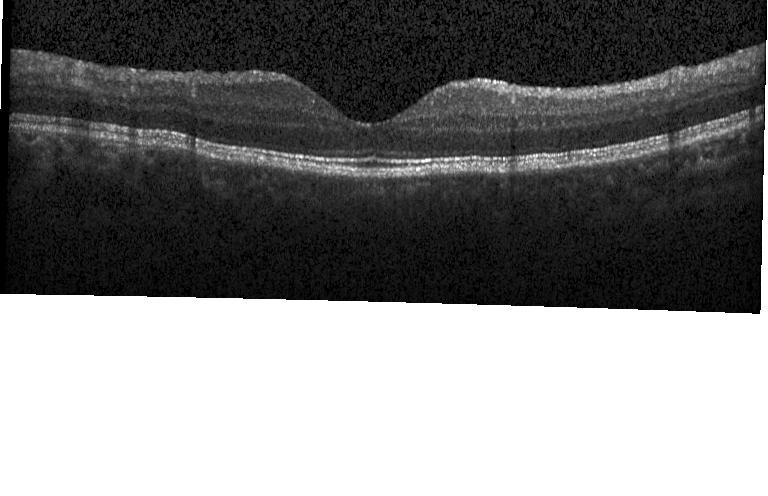

Optical coherence tomography scan · through the macula · Heidelberg Spectralis OCT system.
Diagnosis: no choroidal neovascularization, no diabetic macular edema, and no drusen.